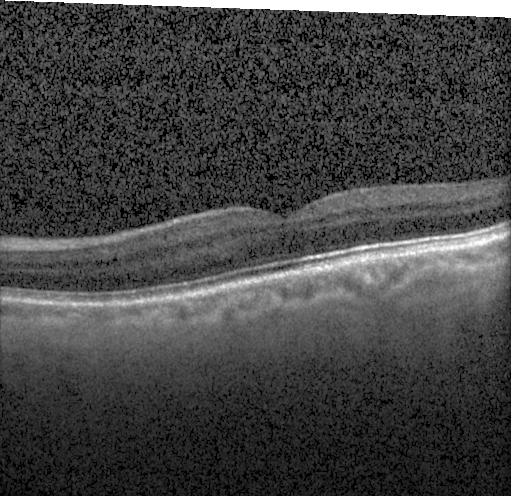

Through the macula; retinal OCT B-scan; SD-OCT; instrument: Heidelberg Spectralis
OCT finding: neither choroidal neovascularization, diabetic macular edema, nor drusen.